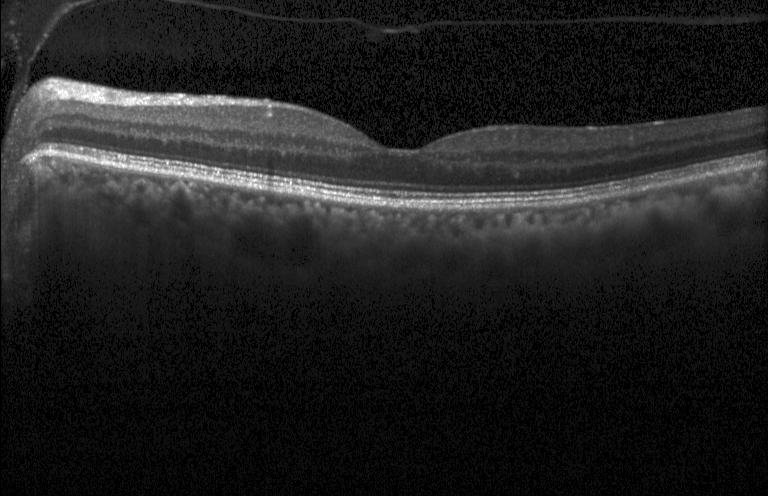
Finding: no evidence of CNV, DME, or drusen.